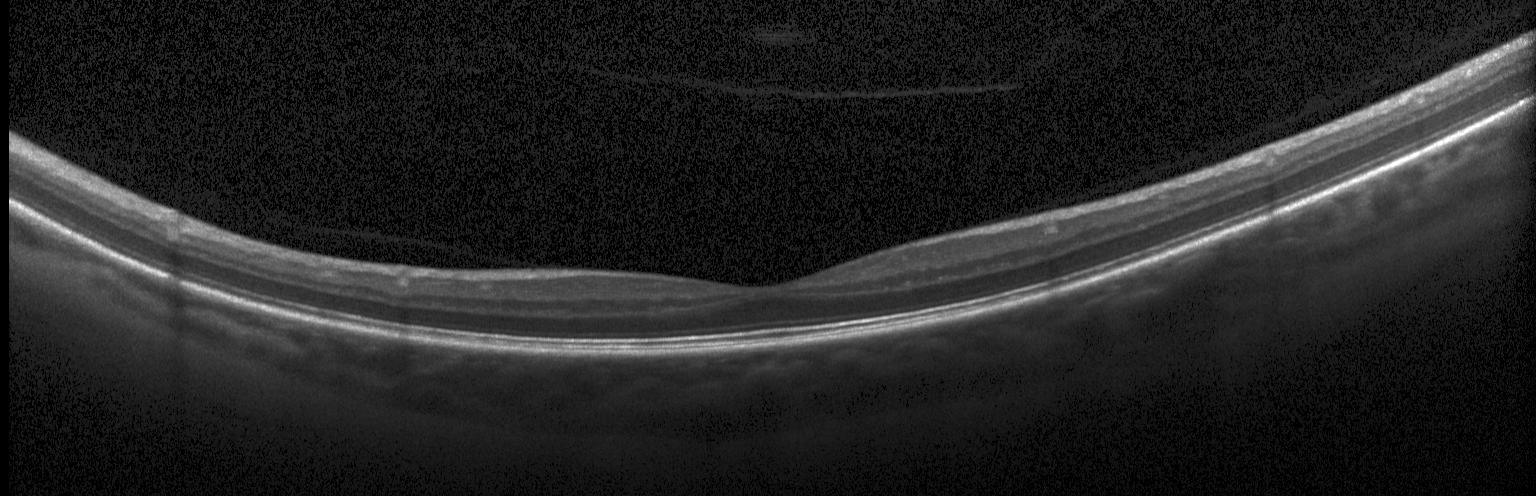
The scan shows no choroidal neovascularization, diabetic macular edema, or drusen.